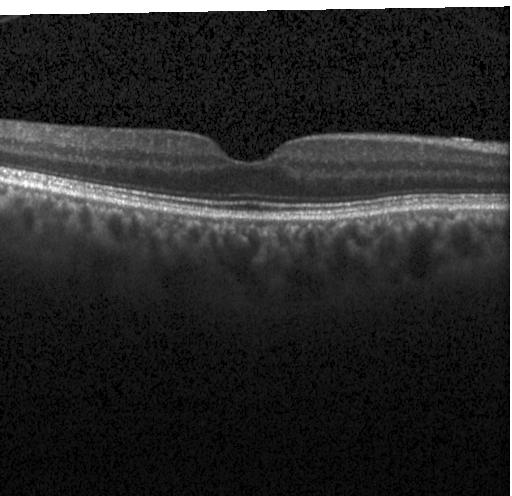

Retinal OCT B-scan, acquired on a Heidelberg Spectralis, macular scan, spectral-domain OCT. Impression: no evidence of CNV, DME, or drusen.